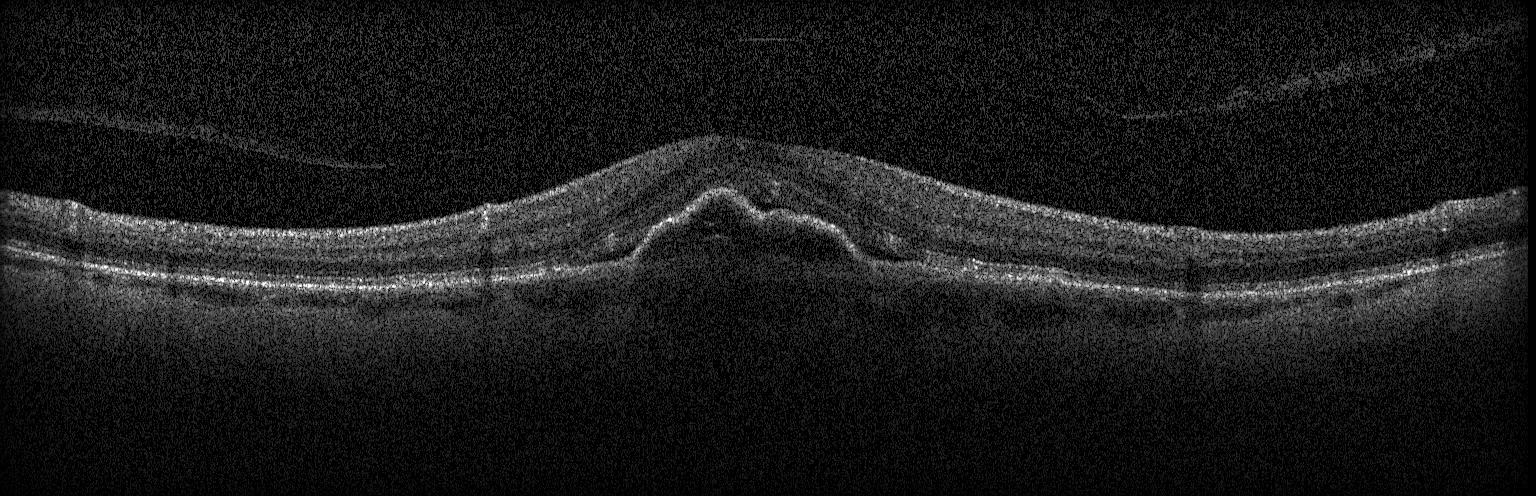

Diagnosis: a choroidal neovascular membrane.